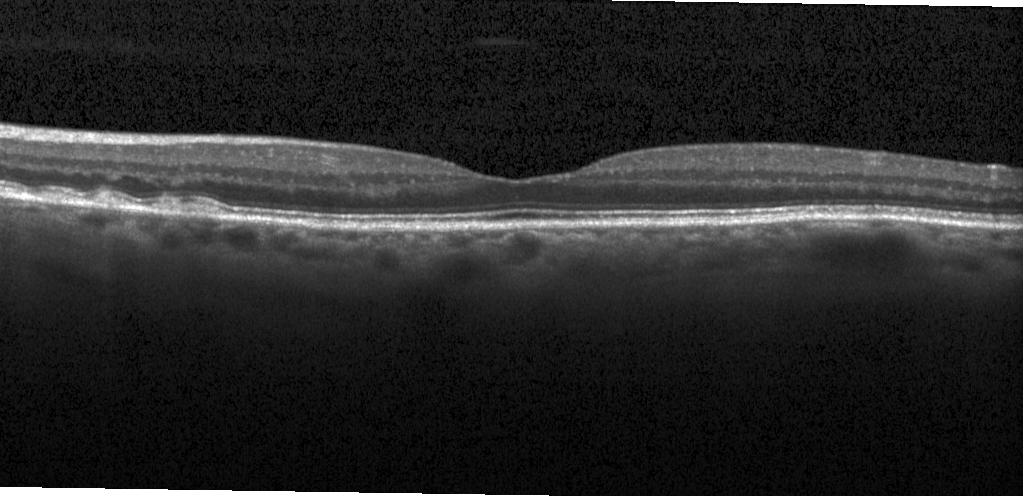 Optical coherence tomography B-scan. Finding: sub-RPE drusenoid deposits.